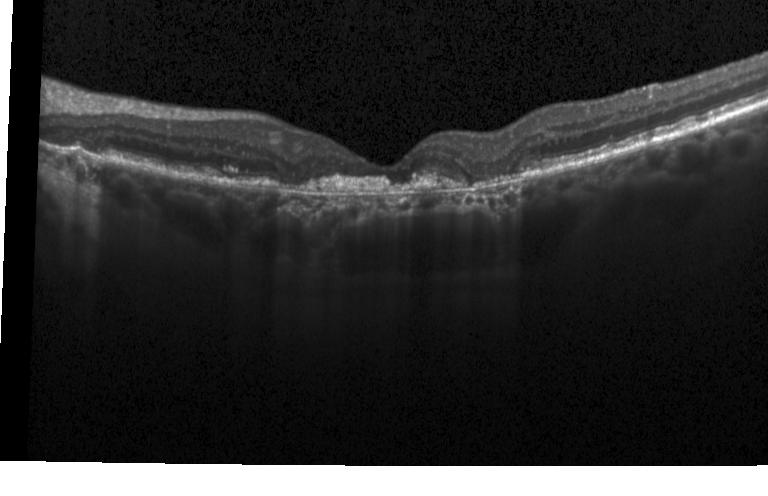

Diagnosis: a choroidal neovascular membrane.